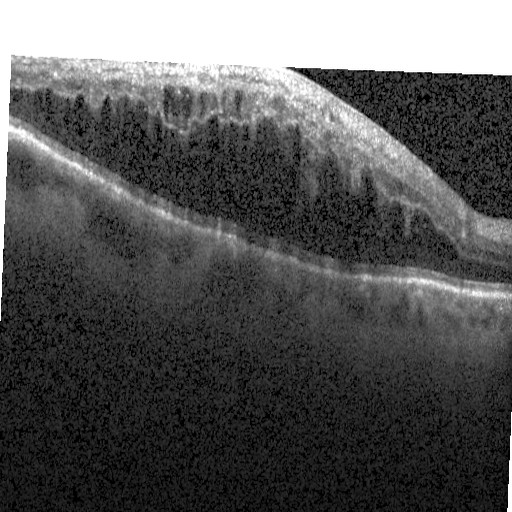
Retinal OCT cross-section. SD-OCT. Acquired on a Heidelberg Spectralis — OCT finding: DME.